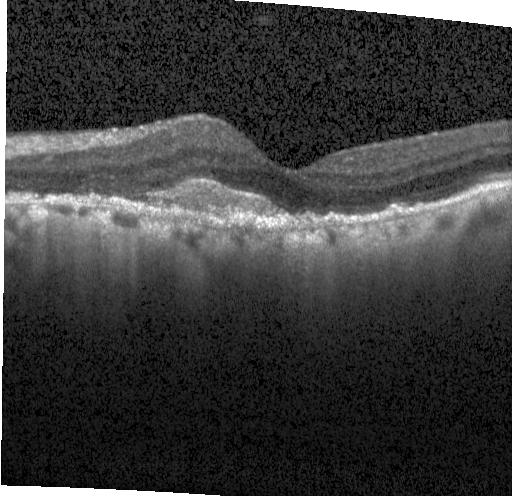 Retinal OCT cross-section — Diagnosis: choroidal neovascularization.